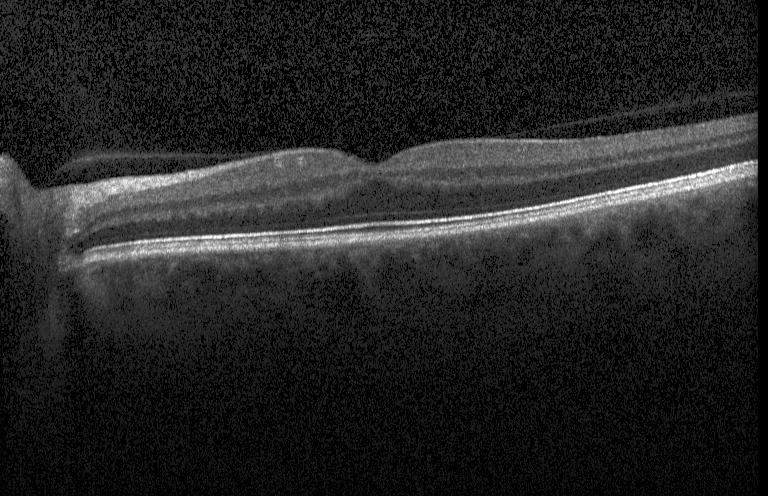
Optical coherence tomography B-scan. Macular OCT: no choroidal neovascularization, no diabetic macular edema, and no drusen.